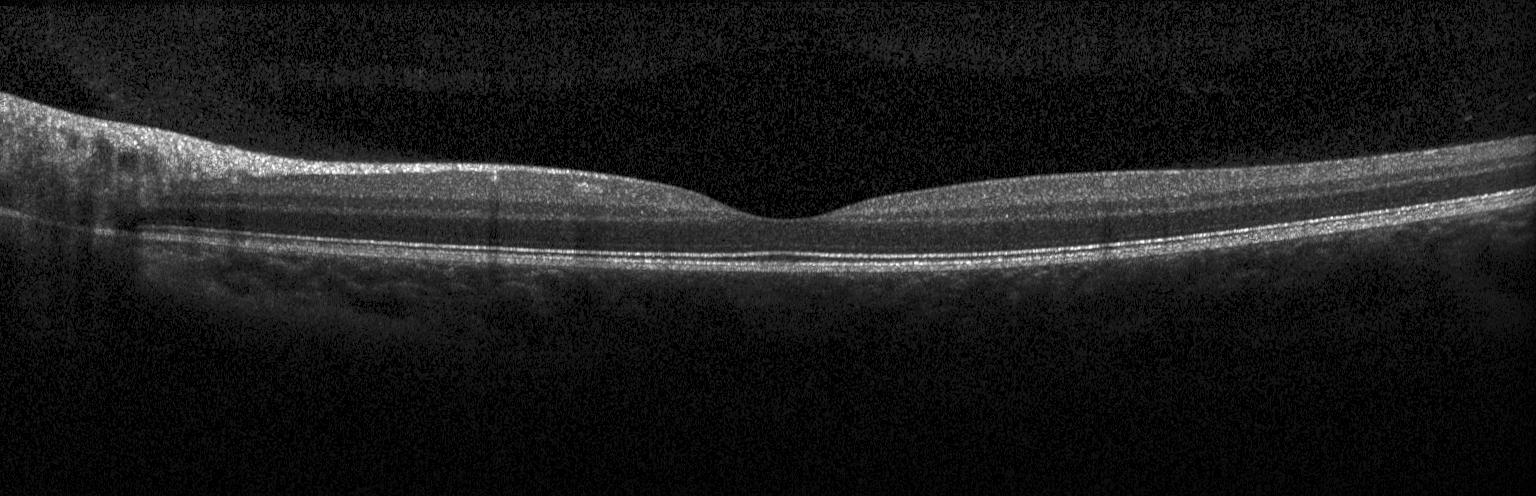 Retinal OCT B-scan. Dx: neither CNV, DME, nor drusen.